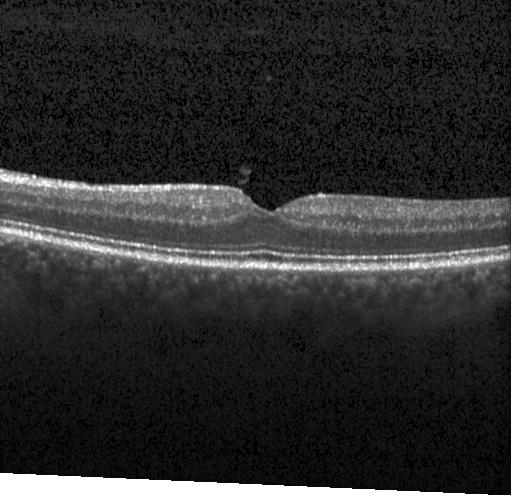
Optical coherence tomography scan.
This B-scan demonstrates no choroidal neovascularization, no diabetic macular edema, and no drusen.